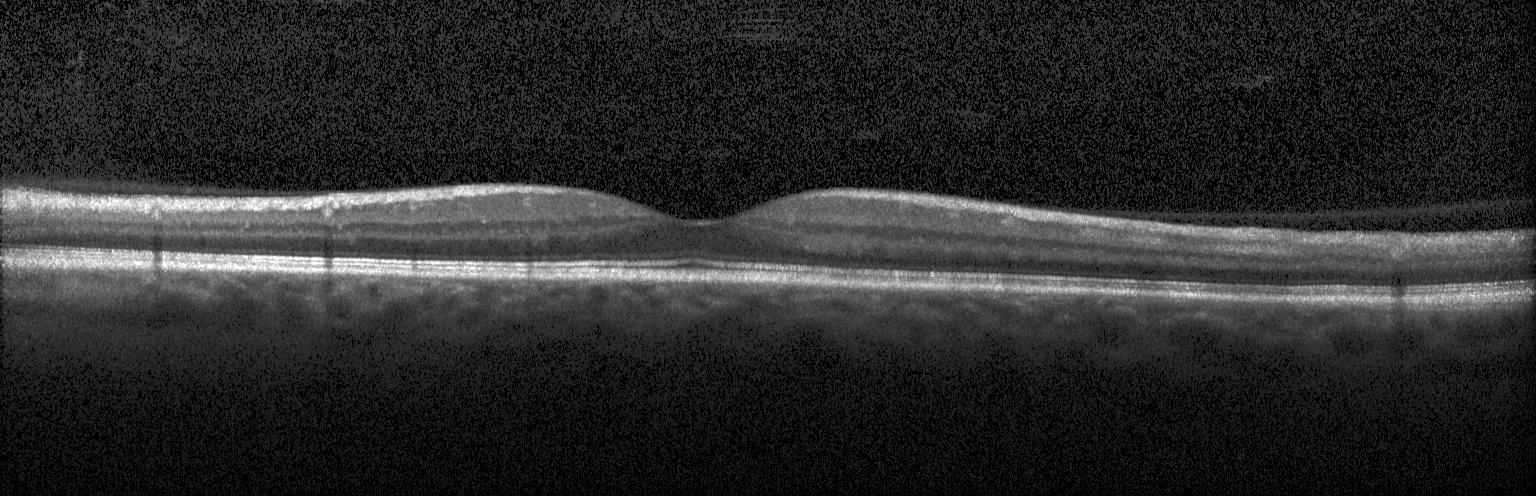
Finding: no CNV, DME, or drusen.